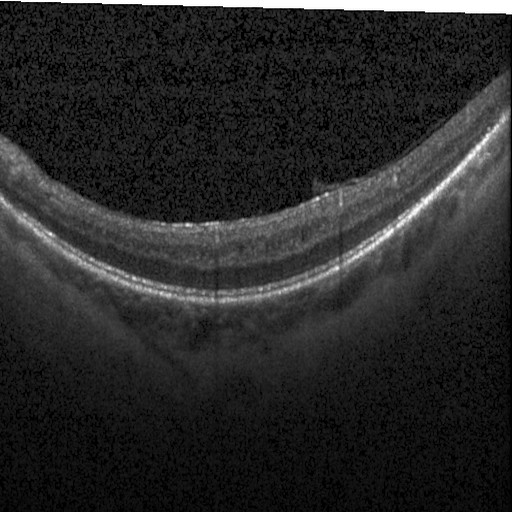 Finding: diabetic macular edema.